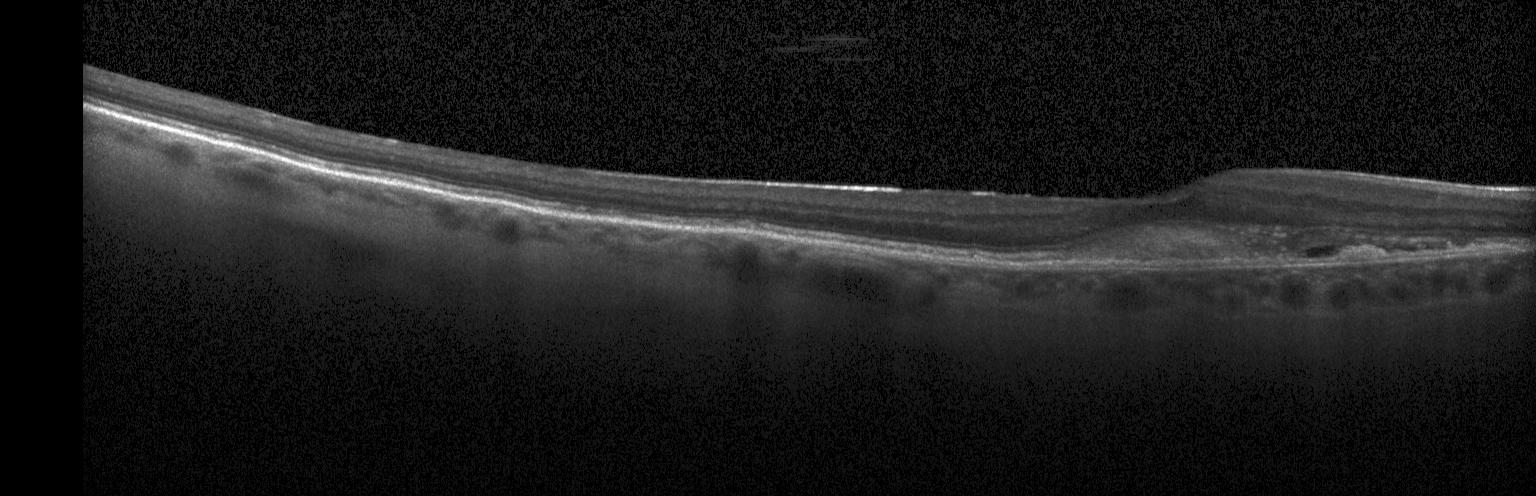 Retinal OCT cross-section; acquired on a Heidelberg Spectralis; through the macula — Impression: CNV.